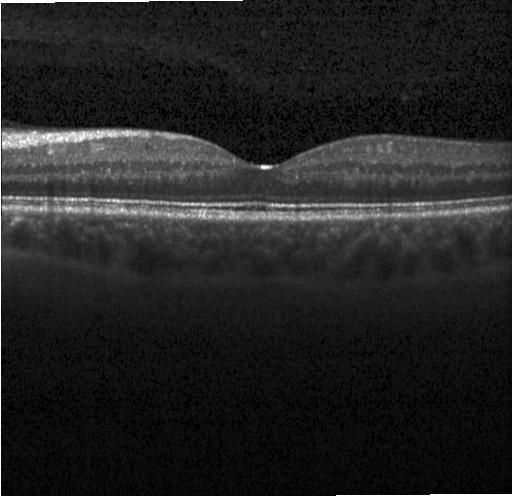

Finding: neither CNV, DME, nor drusen.